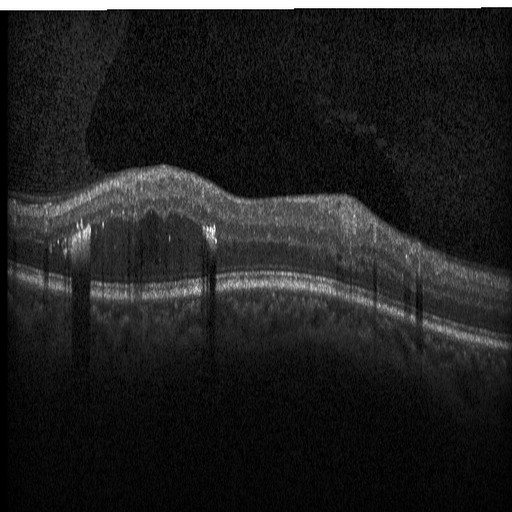
Diagnosis: diabetic macular edema.